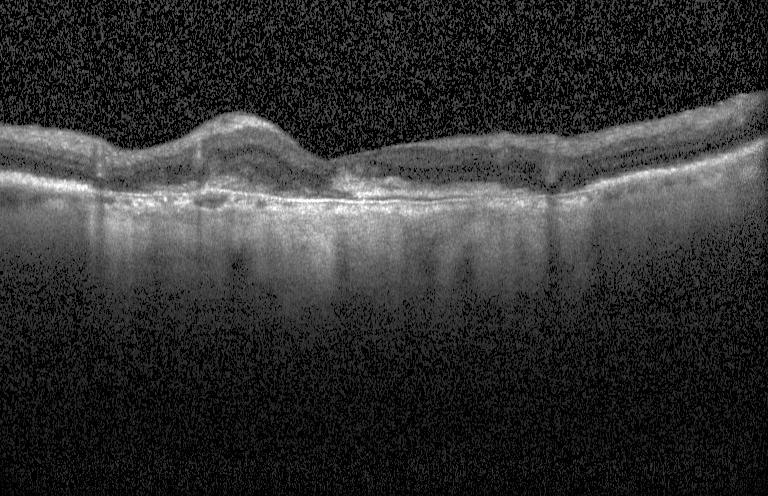
Diagnosis: choroidal neovascularization.